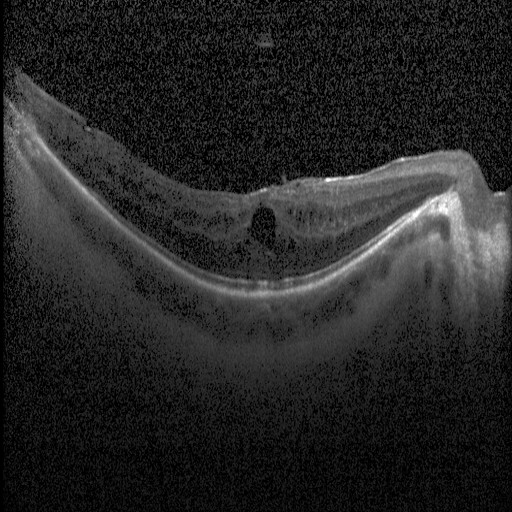

OCT line scan; acquired on a Heidelberg Spectralis; spectral-domain optical coherence tomography; horizontal scan through the fovea. Macular OCT: DME.